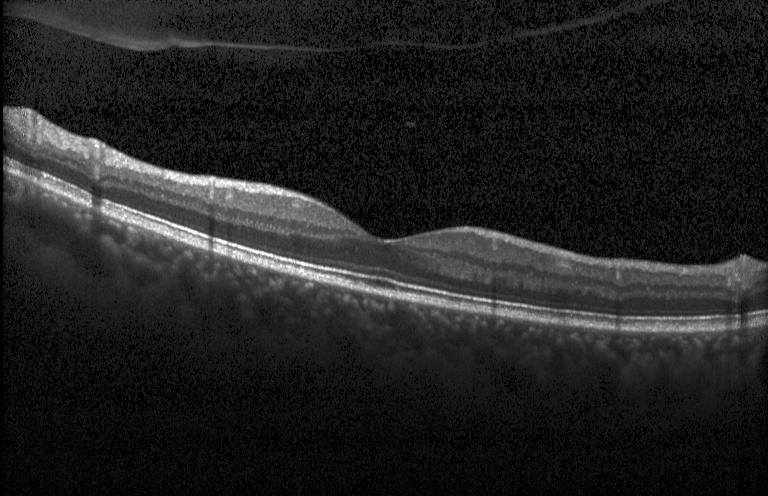 Diagnosis: no choroidal neovascularization, no diabetic macular edema, and no drusen.